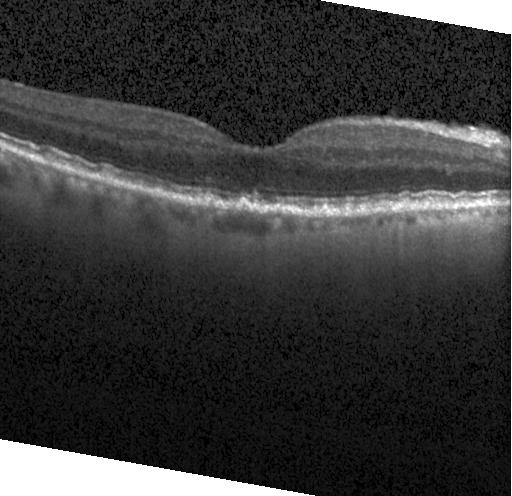

The scan shows drusen.